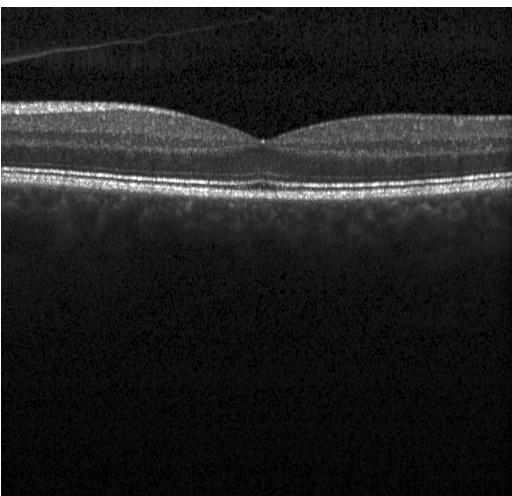
Heidelberg Spectralis OCT system · optical coherence tomography B-scan
No evidence of choroidal neovascularization, diabetic macular edema, or drusen.